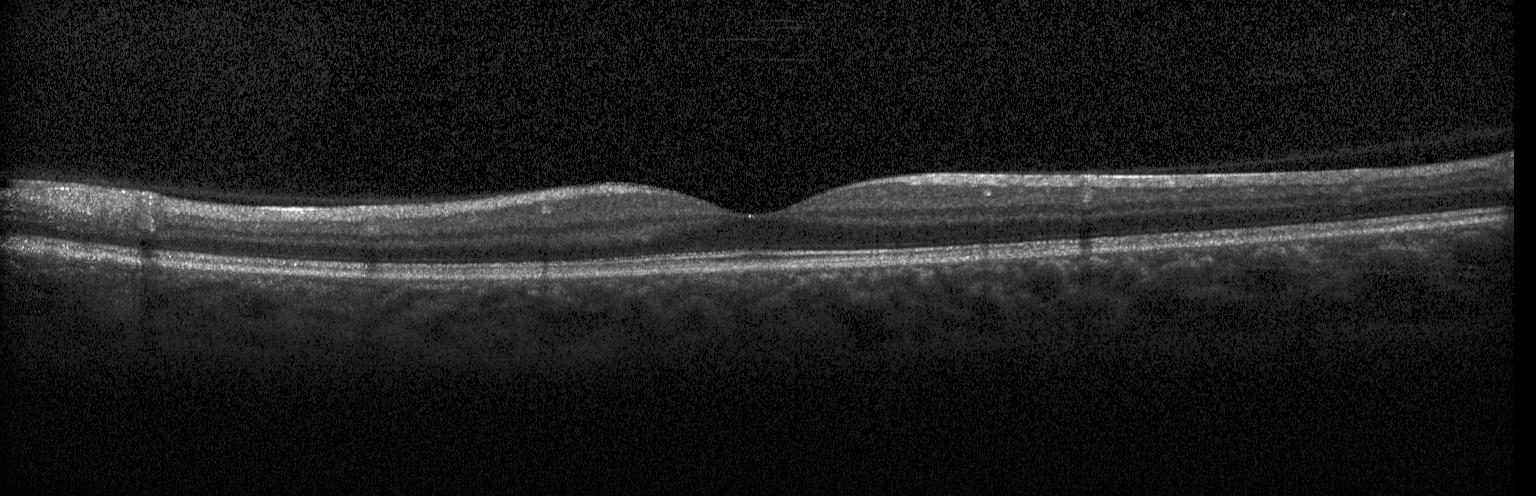
Instrument: Heidelberg Spectralis, retinal OCT B-scan — Diagnosis: no evidence of choroidal neovascularization, diabetic macular edema, or drusen.